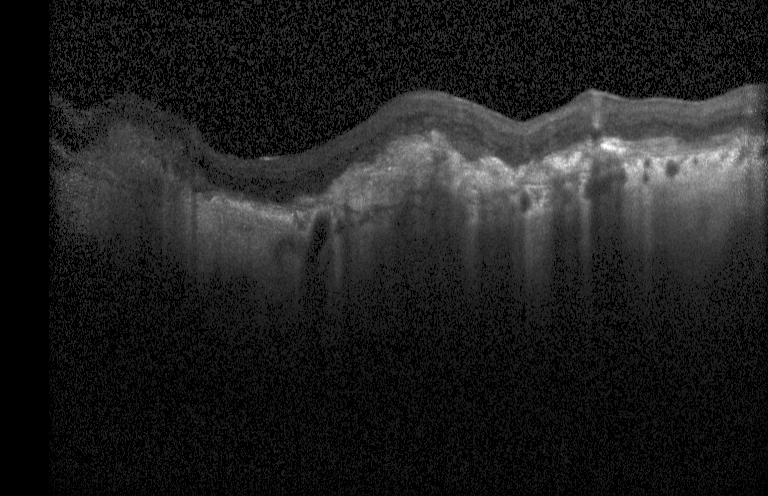

Acquired on a Heidelberg Spectralis · retinal OCT cross-section.
Diagnosis: choroidal neovascularization (CNV).